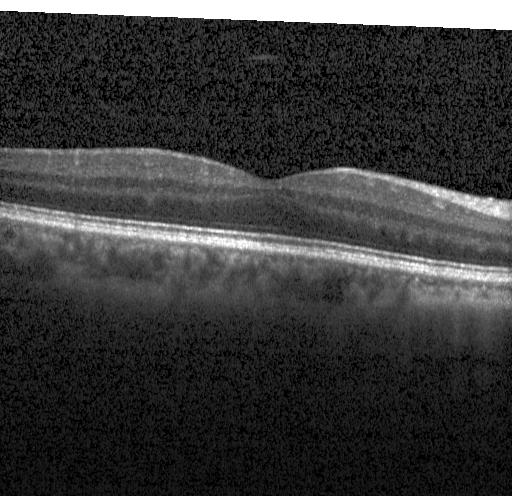 Retinal OCT B-scan — This B-scan demonstrates no CNV, no DME, and no drusen.